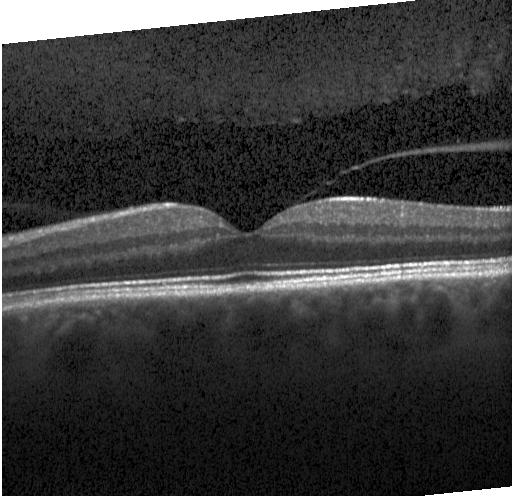

OCT B-scan.
No choroidal neovascularization, diabetic macular edema, or drusen.